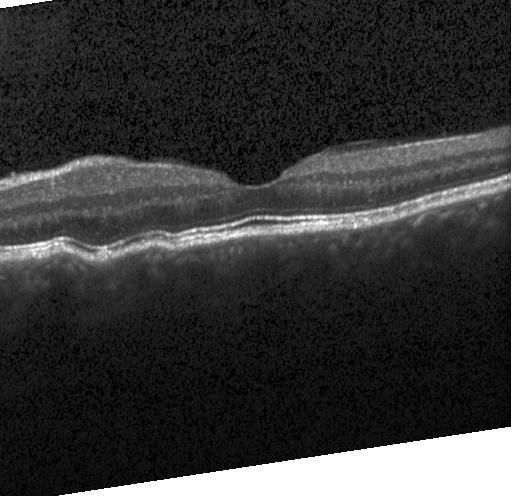 Finding: neither choroidal neovascularization, diabetic macular edema, nor drusen.